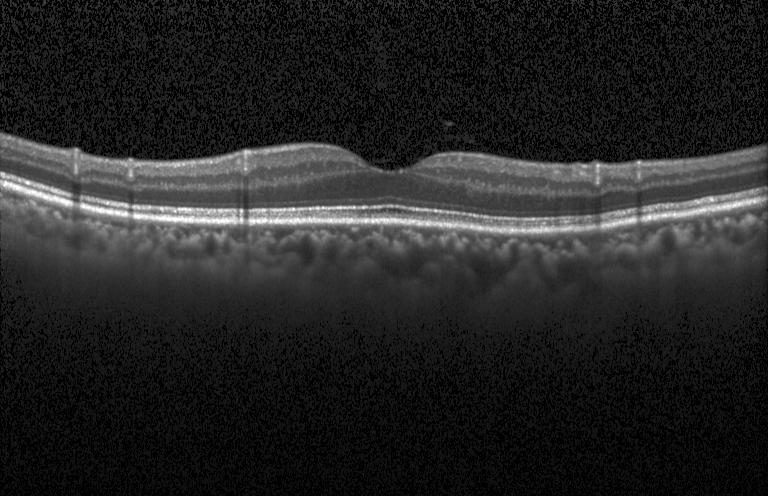
OCT scan showing no choroidal neovascularization, diabetic macular edema, or drusen.